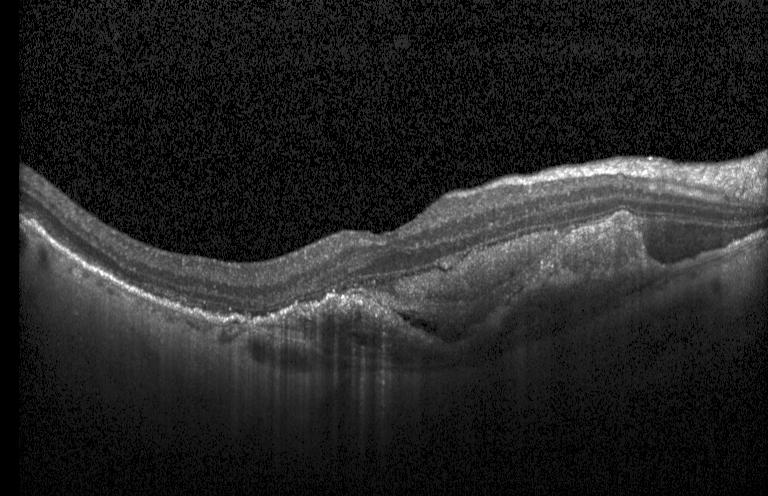 Optical coherence tomography B-scan, Heidelberg Spectralis OCT system. Assessment: CNV.